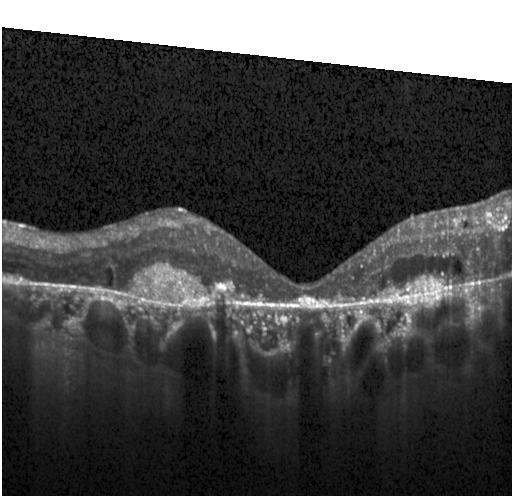 Macular scan, SD-OCT, OCT B-scan.
The scan shows choroidal neovascularization (CNV).